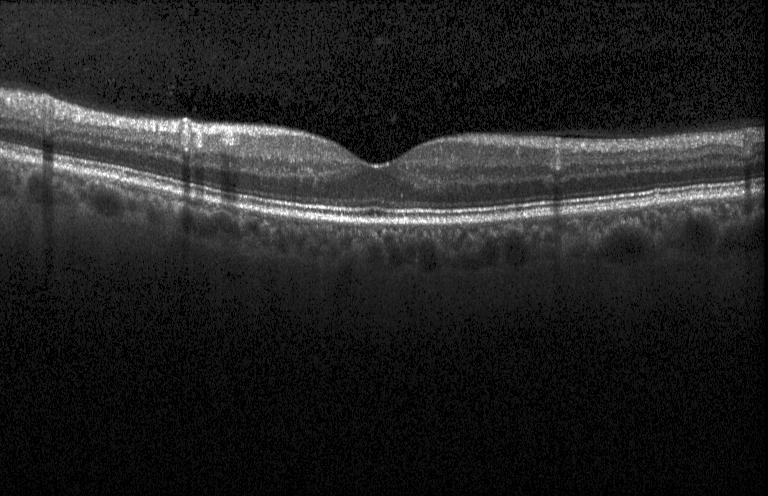
Heidelberg Spectralis OCT system; retinal OCT B-scan.
This B-scan demonstrates no choroidal neovascularization, no diabetic macular edema, and no drusen.